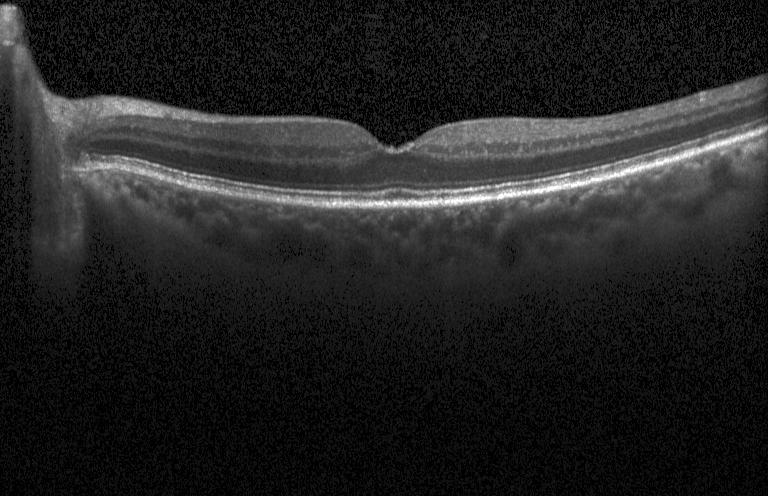
No CNV, no DME, and no drusen.